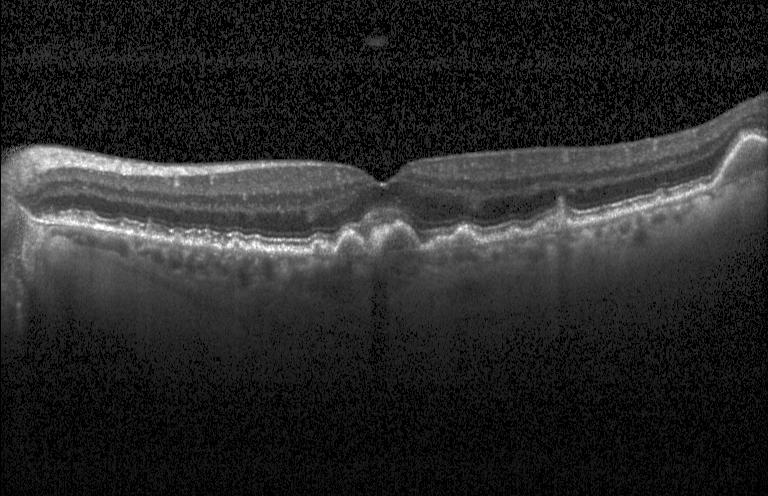
OCT B-scan.
Dx: choroidal neovascularization (CNV).